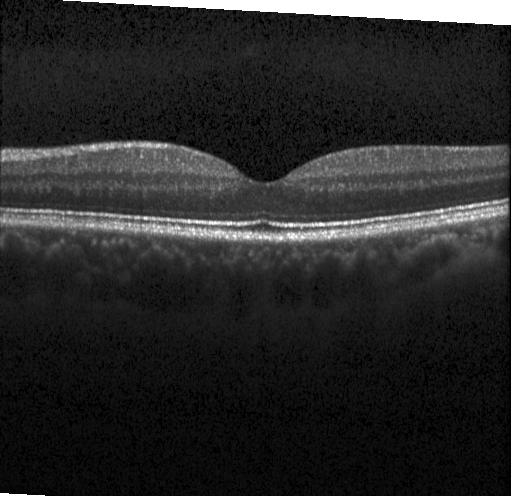
Optical coherence tomography scan — Neither choroidal neovascularization, diabetic macular edema, nor drusen.